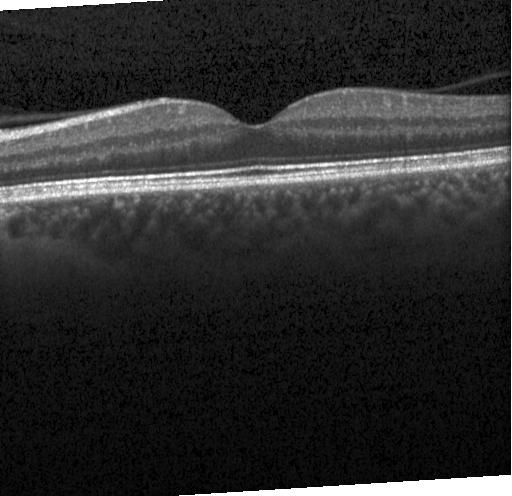 Impression: neither choroidal neovascularization, diabetic macular edema, nor drusen.